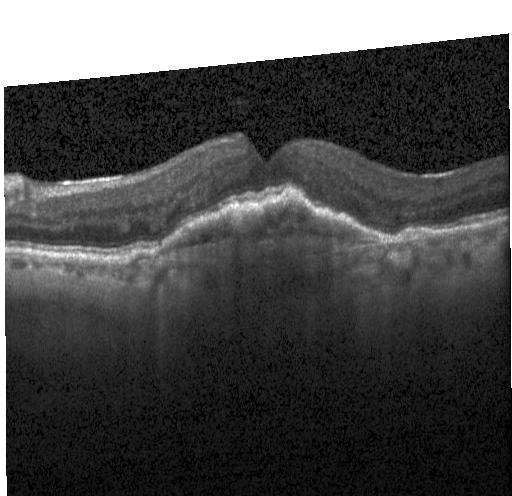 Instrument: Heidelberg Spectralis · retinal OCT cross-section · spectral-domain optical coherence tomography. Diagnosis: a choroidal neovascular membrane.